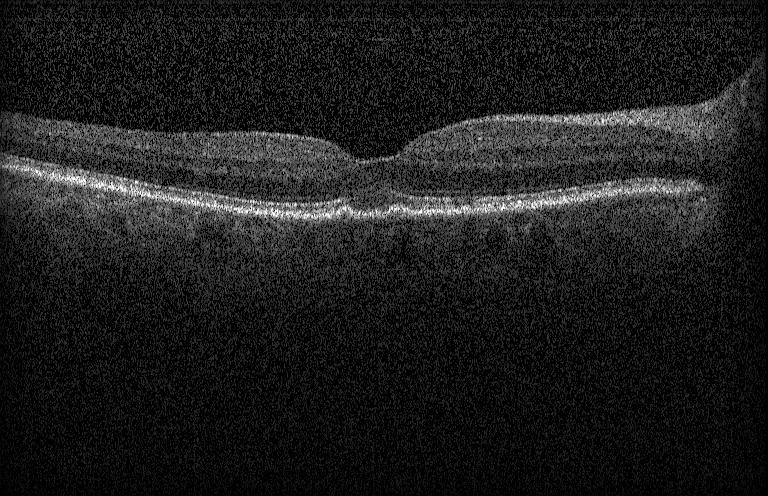 OCT line scan. Heidelberg Spectralis. Fovea-centered.
Diagnosis: sub-RPE drusenoid deposits.